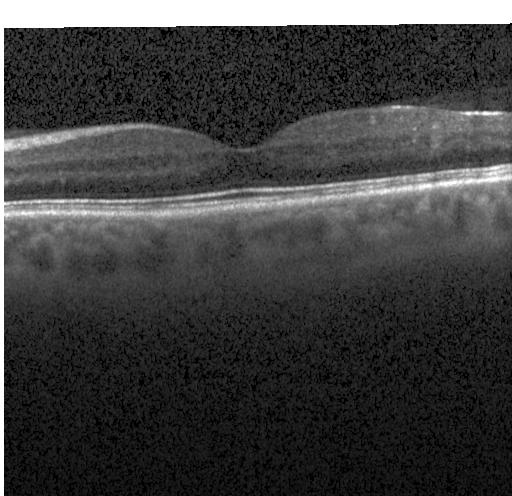

Finding: neither CNV, DME, nor drusen.